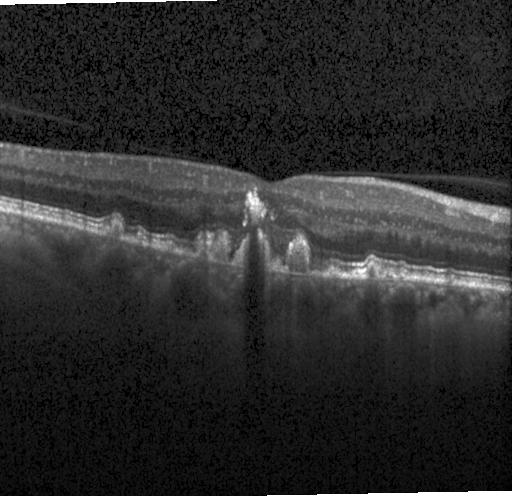

Heidelberg Spectralis · spectral-domain optical coherence tomography · centered on the fovea · retinal OCT B-scan. This B-scan demonstrates CNV.